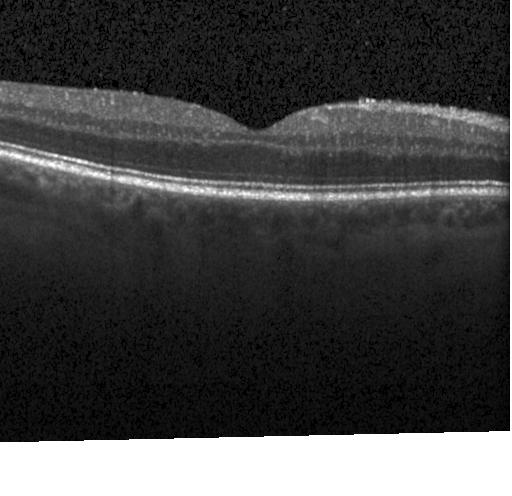 The scan shows no evidence of choroidal neovascularization, diabetic macular edema, or drusen.